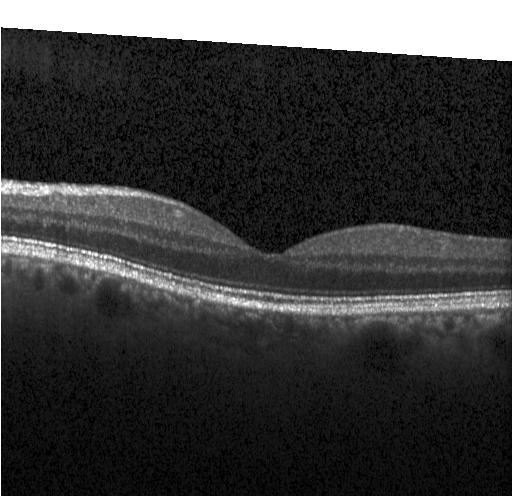 OCT line scan.
Diagnosis: no choroidal neovascularization, diabetic macular edema, or drusen.